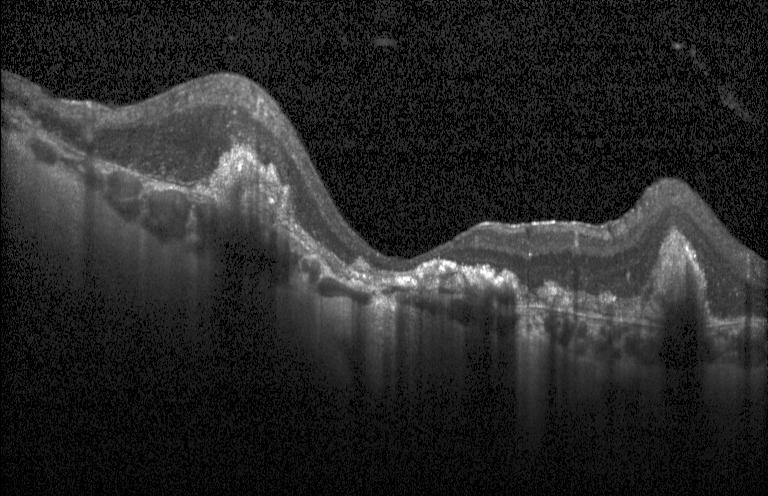

OCT B-scan, SD-OCT, centered on the fovea.
Diagnosis: CNV.